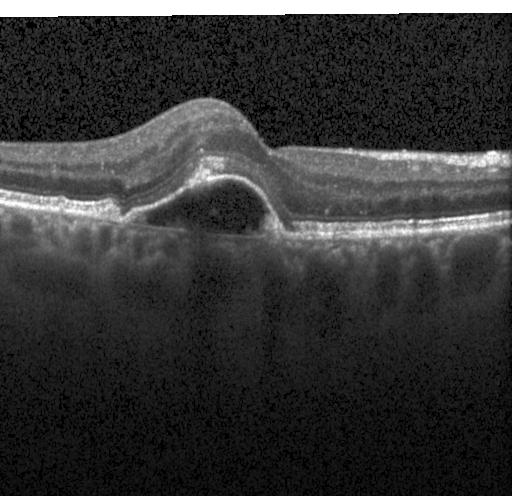
Diagnosis: choroidal neovascularization.